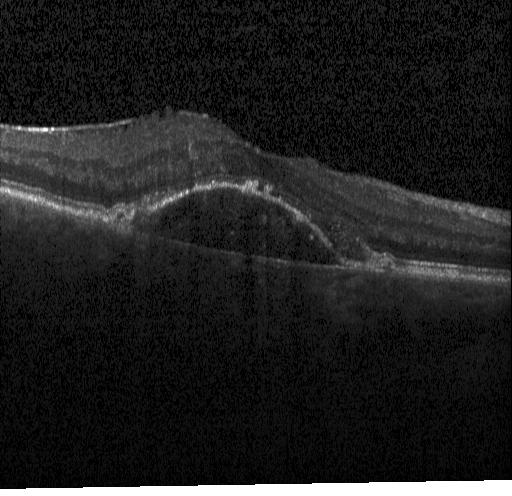 Macular OCT demonstrating CNV.